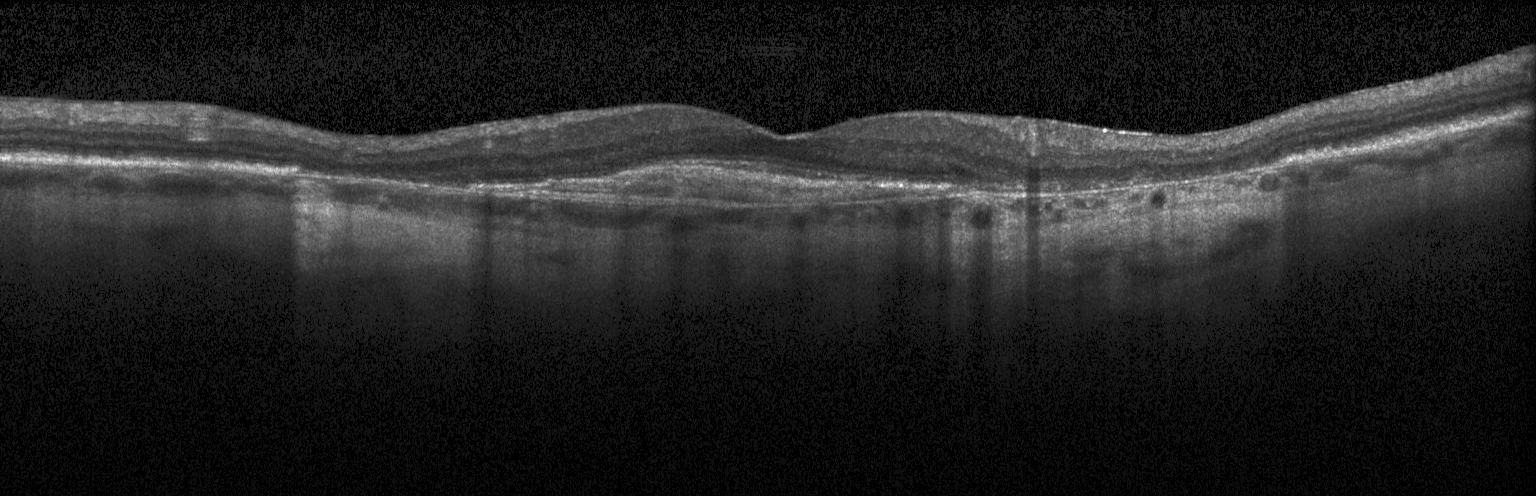

Diagnosis: a choroidal neovascular membrane.